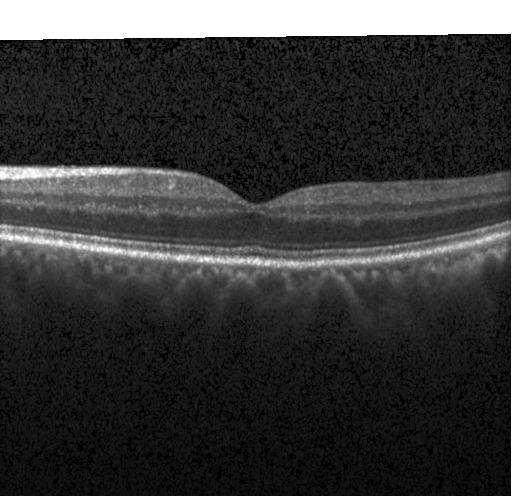 OCT line scan.
Assessment: no evidence of choroidal neovascularization, diabetic macular edema, or drusen.